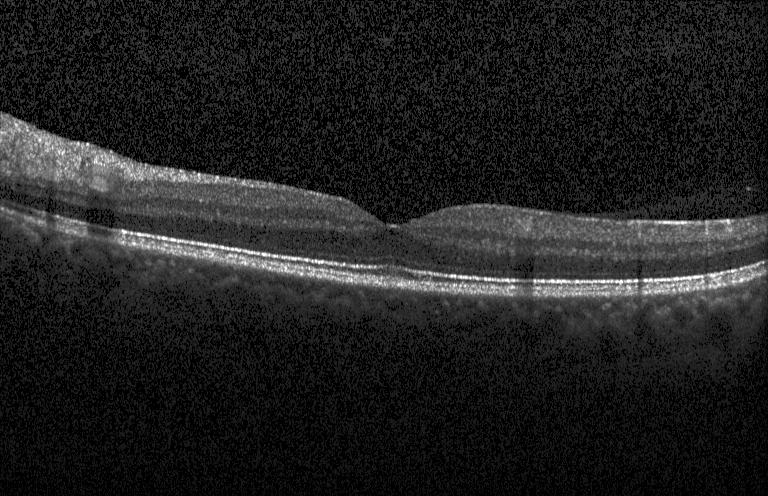 OCT line scan, Heidelberg Spectralis OCT system, macular scan — Finding: neither choroidal neovascularization, diabetic macular edema, nor drusen.